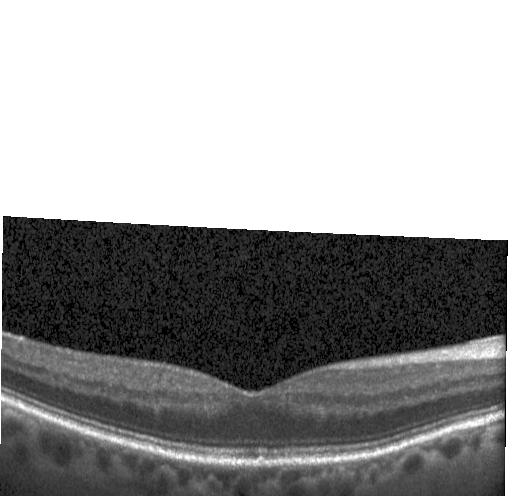 Spectral-domain OCT · retinal OCT B-scan · centered on the fovea. This B-scan demonstrates no evidence of CNV, DME, or drusen.